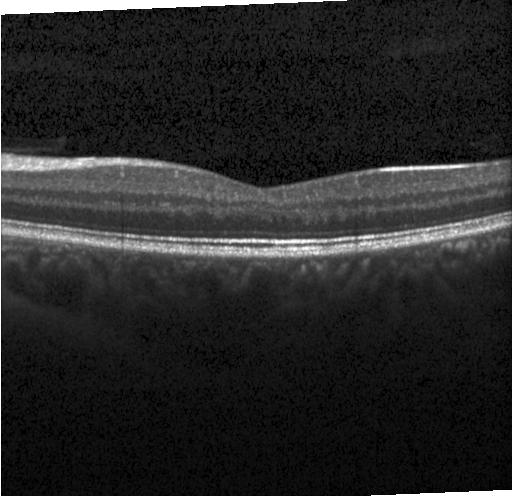
The scan shows neither CNV, DME, nor drusen.